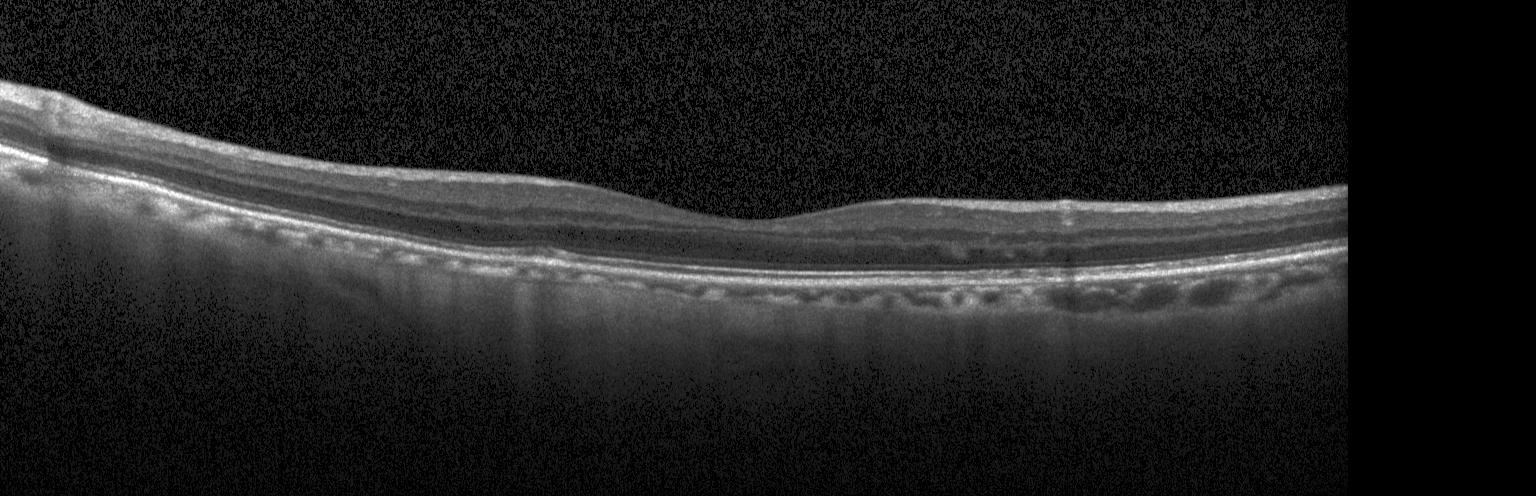
Spectral-domain optical coherence tomography, retinal OCT cross-section — Diagnosis: no choroidal neovascularization, no diabetic macular edema, and no drusen.